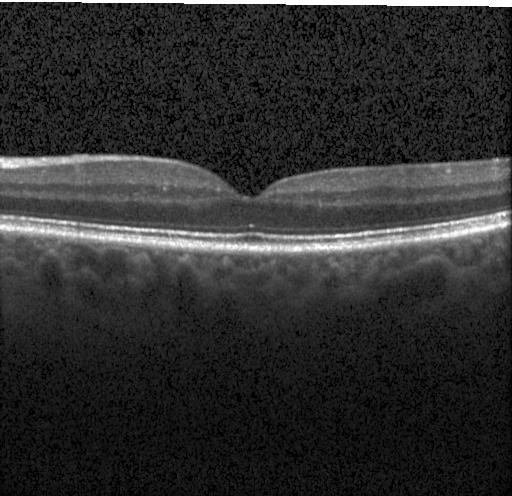
OCT B-scan showing no choroidal neovascularization, no diabetic macular edema, and no drusen.